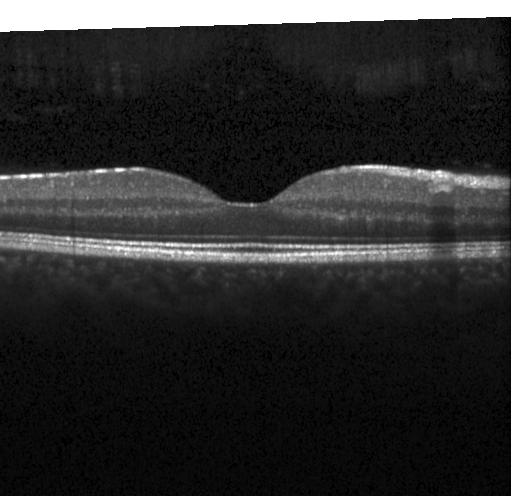
Fovea-centered · retinal OCT B-scan.
Impression: no CNV, no DME, and no drusen.